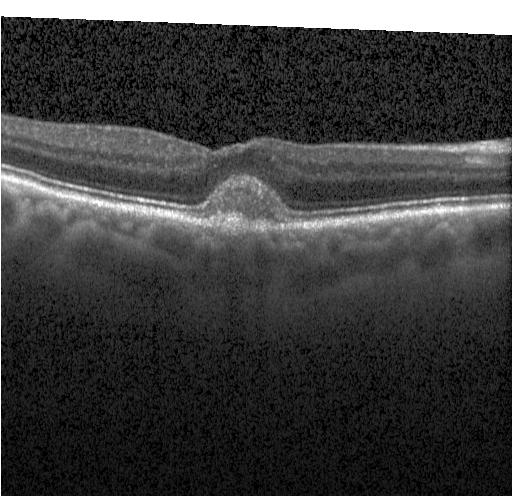
OCT finding: CNV.